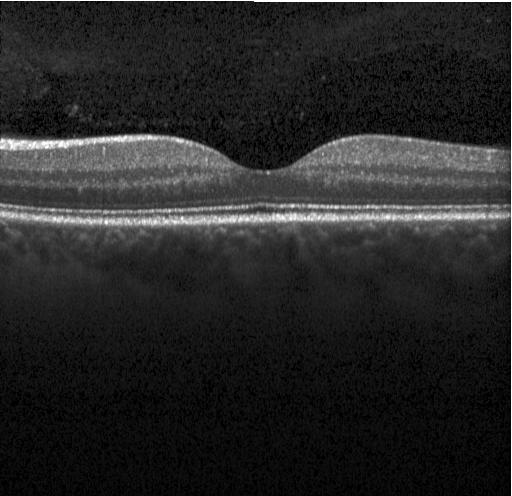 Horizontal scan through the fovea. Instrument: Heidelberg Spectralis. OCT line scan.
Macular OCT: no evidence of choroidal neovascularization, diabetic macular edema, or drusen.